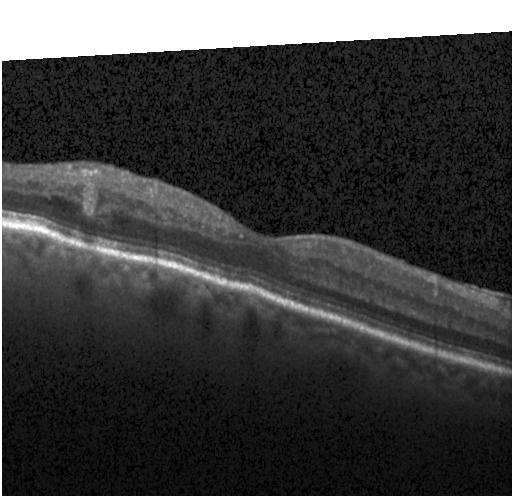 Neither choroidal neovascularization, diabetic macular edema, nor drusen.